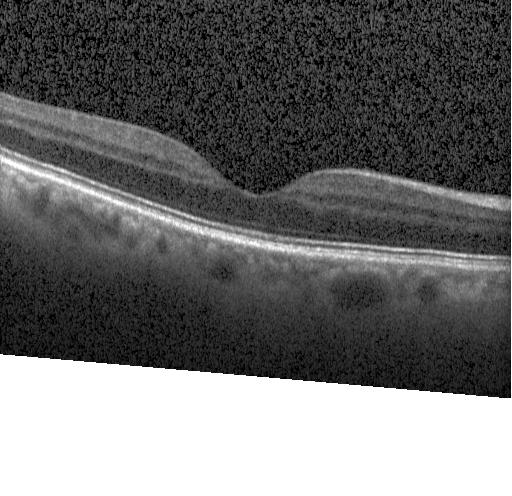

OCT finding: no choroidal neovascularization, no diabetic macular edema, and no drusen.